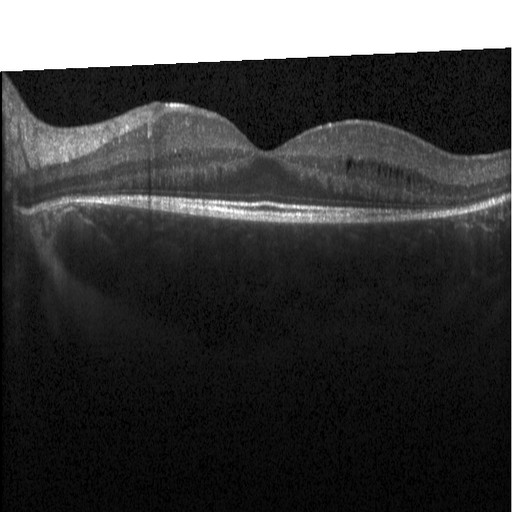
Finding: diabetic macular edema.